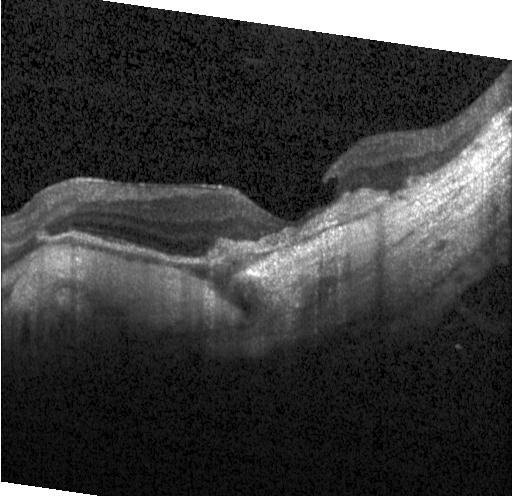
Optical coherence tomography B-scan. Finding: a choroidal neovascular membrane.